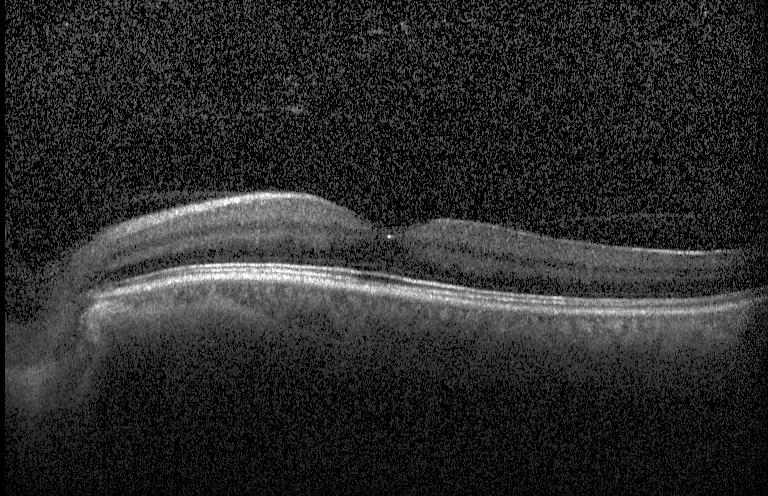 Finding: no evidence of choroidal neovascularization, diabetic macular edema, or drusen.